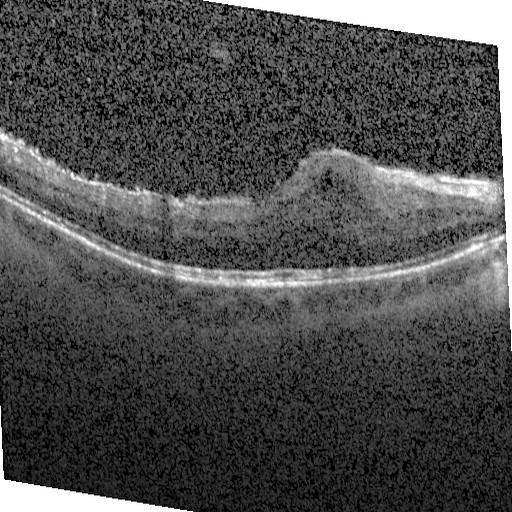 Retinal OCT cross-section
Assessment: diabetic macular edema (DME).